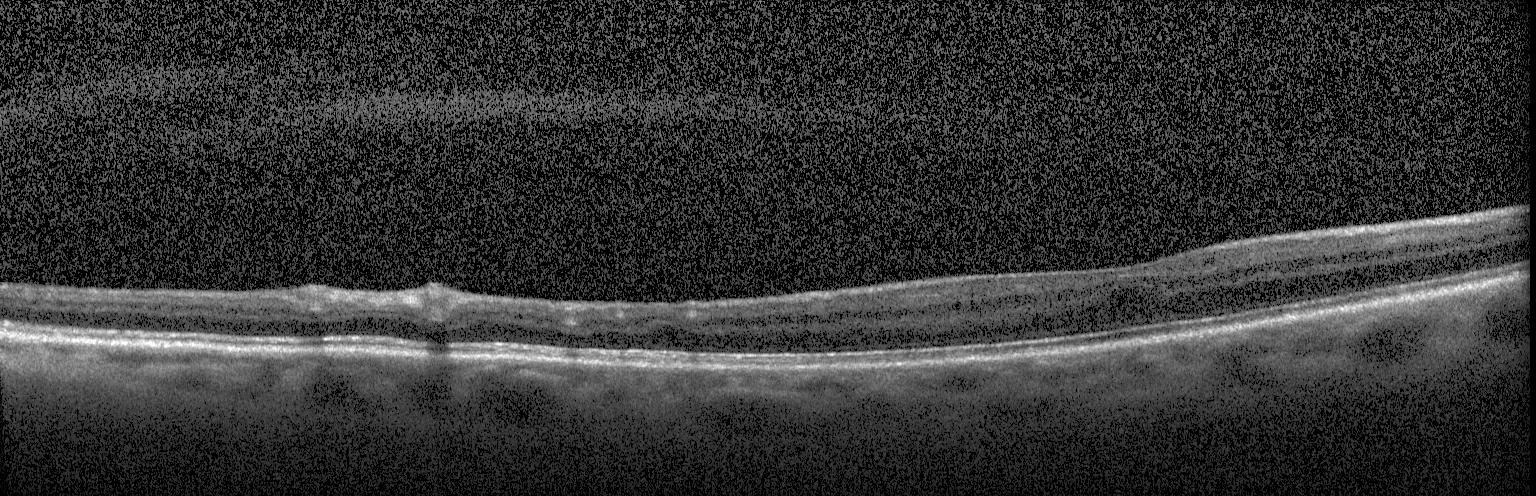
Retinal OCT cross-section, through the macula
Impression: no choroidal neovascularization, no diabetic macular edema, and no drusen.